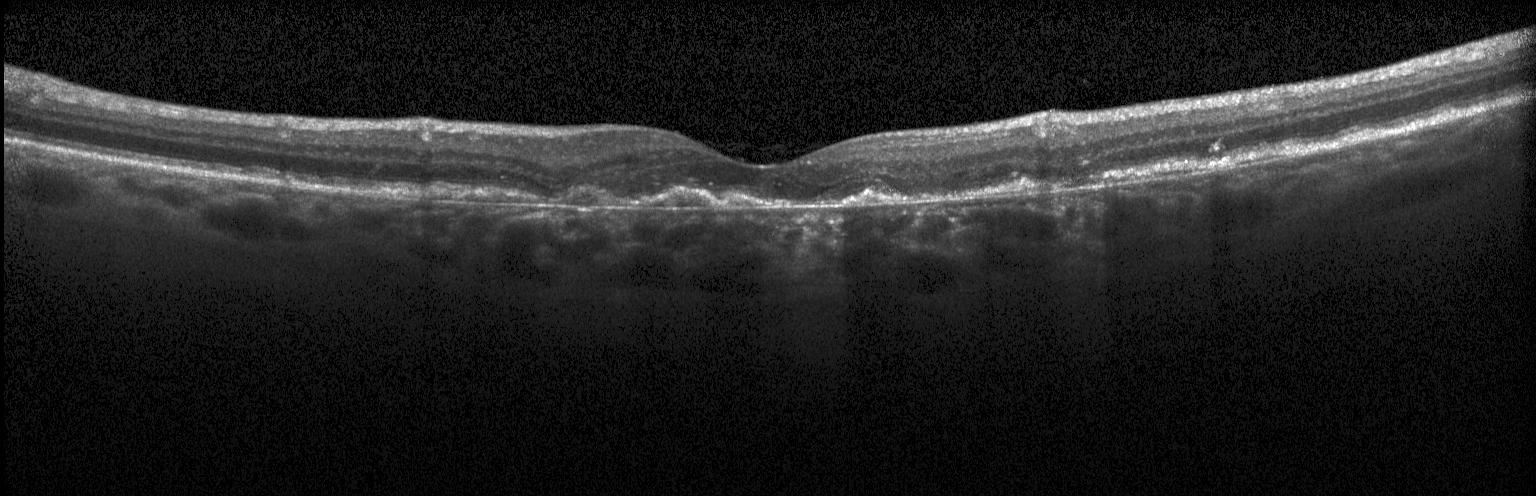

OCT scan showing a choroidal neovascular membrane.